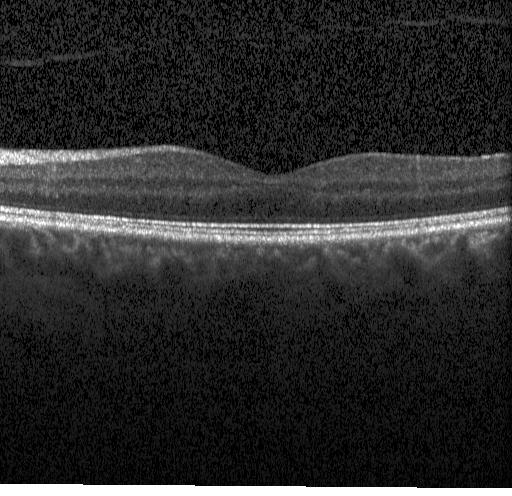

No choroidal neovascularization, diabetic macular edema, or drusen.